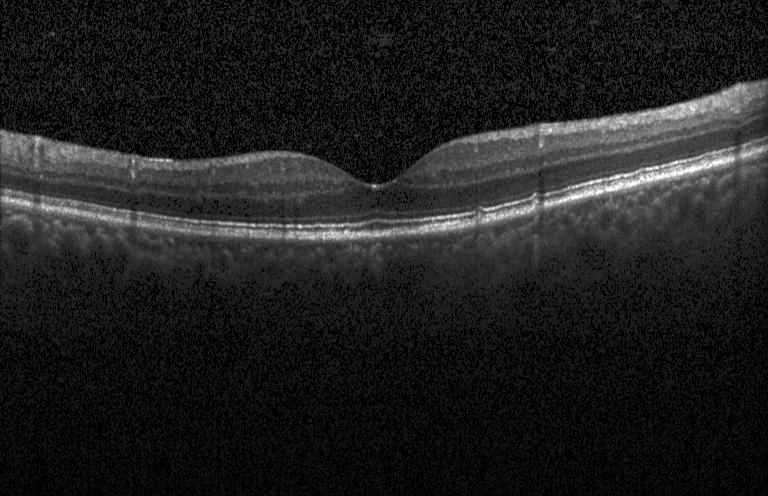

Through the macula, spectral-domain OCT, optical coherence tomography scan — Assessment: drusen.